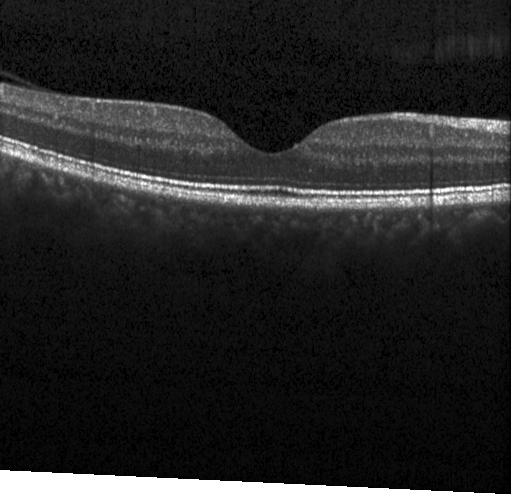
Optical coherence tomography scan — Assessment: no choroidal neovascularization, no diabetic macular edema, and no drusen.